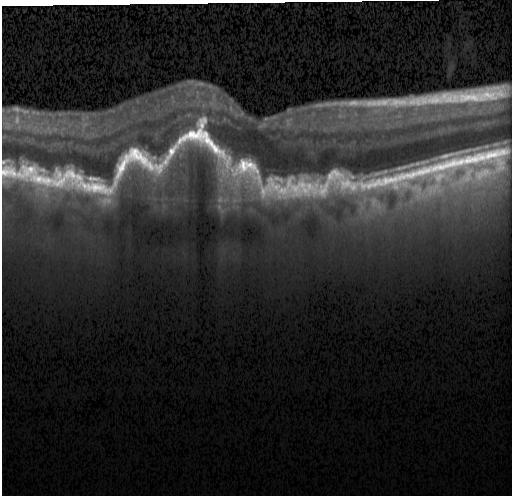
Spectral-domain OCT B-scan: CNV.